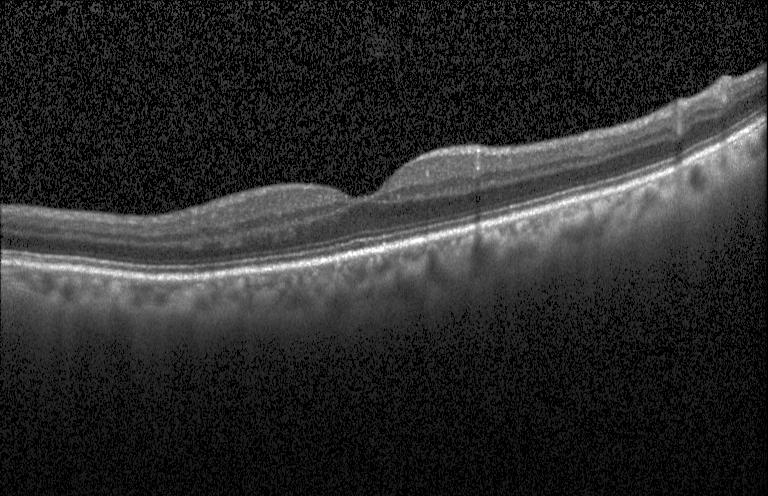
Retinal OCT B-scan.
Diagnosis: neither choroidal neovascularization, diabetic macular edema, nor drusen.